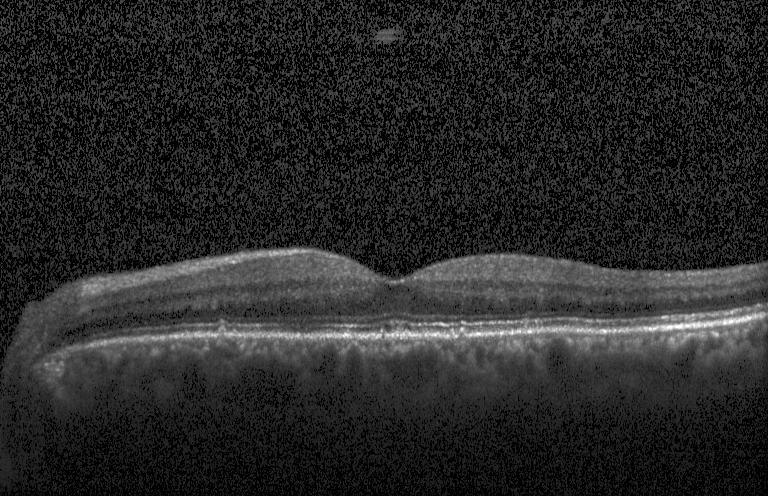 Horizontal scan through the fovea, OCT line scan. Impression: multiple drusen.